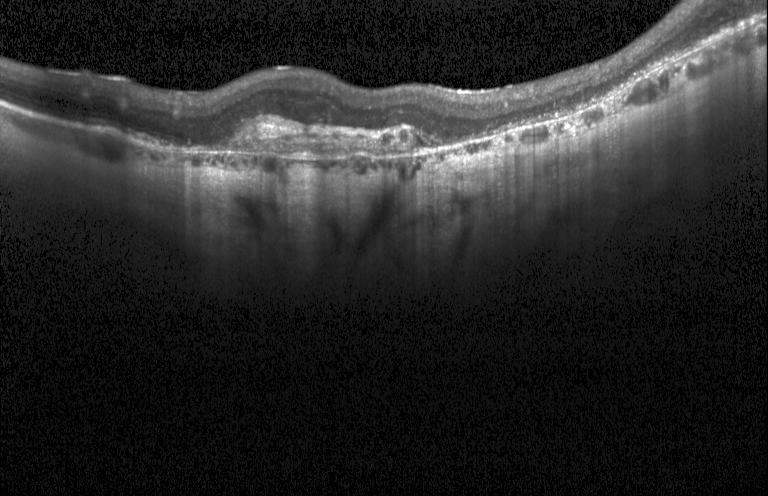
Heidelberg Spectralis OCT system, retinal OCT cross-section, through the macula
Macular OCT: choroidal neovascularization (CNV).